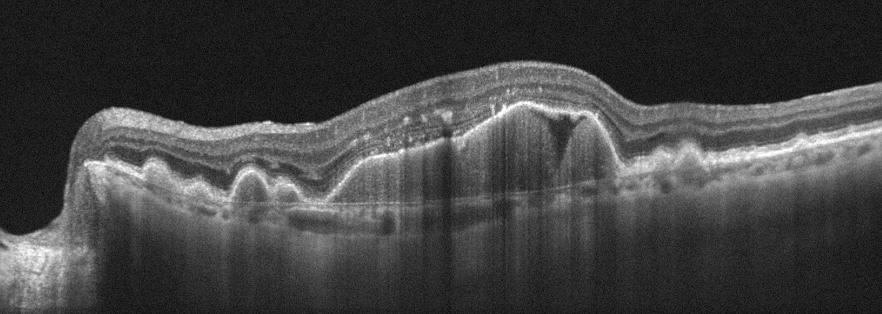

Retinal OCT cross-section showing age-related macular degeneration.